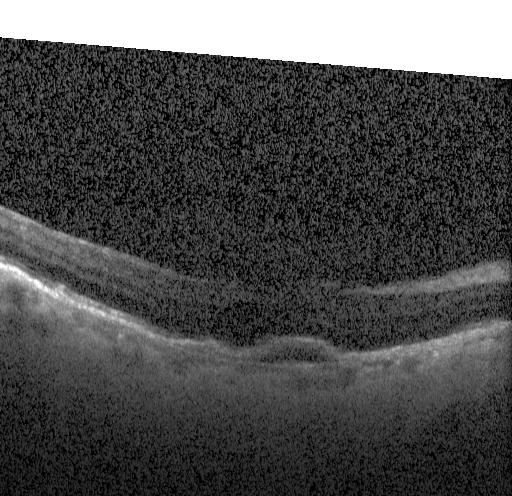 Heidelberg Spectralis; optical coherence tomography scan; spectral-domain OCT; centered on the fovea — OCT finding: choroidal neovascularization.